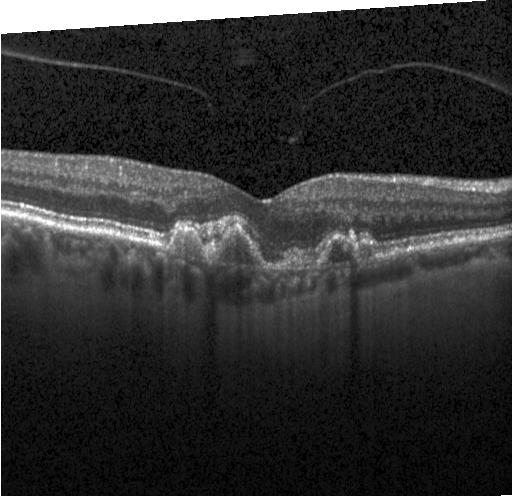

Diagnosis: a choroidal neovascular membrane.